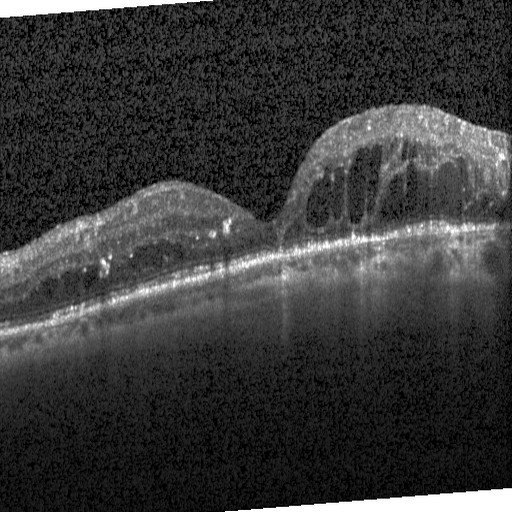

OCT line scan — Diagnosis: DME.